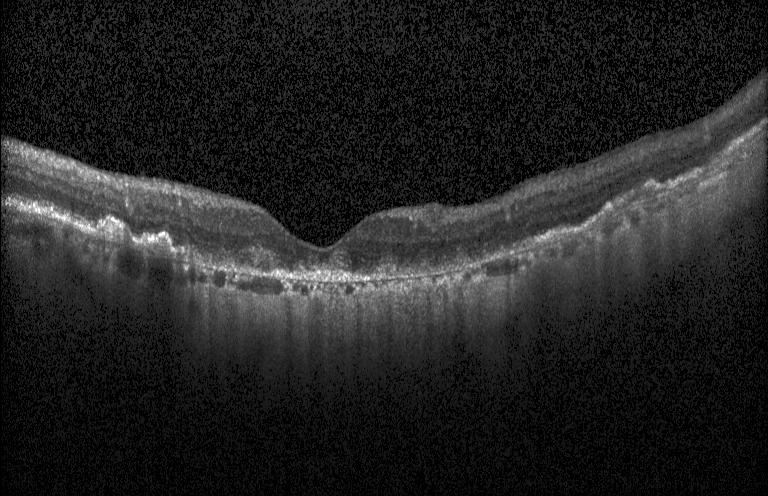 Optical coherence tomography B-scan — Diagnosis: a choroidal neovascular membrane.